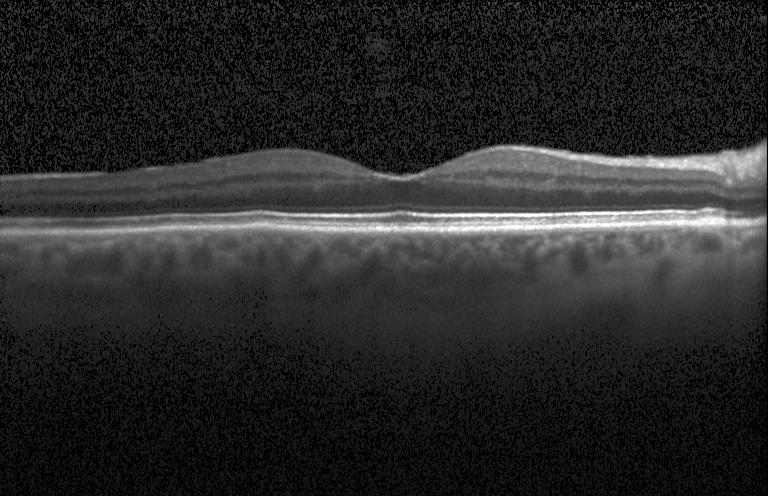

Acquired on a Heidelberg Spectralis; horizontal scan through the fovea; optical coherence tomography B-scan — Impression: no choroidal neovascularization, no diabetic macular edema, and no drusen.